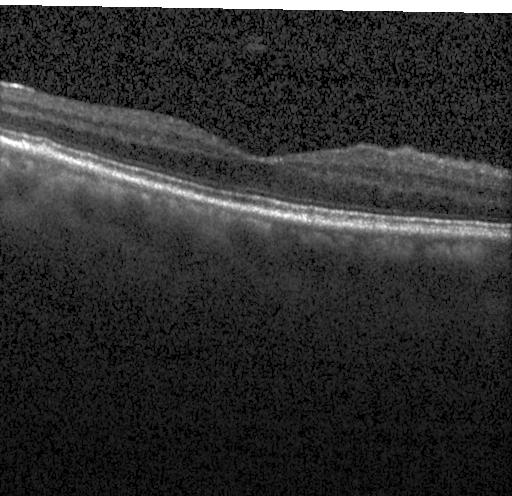
OCT line scan — Assessment: no choroidal neovascularization, diabetic macular edema, or drusen.